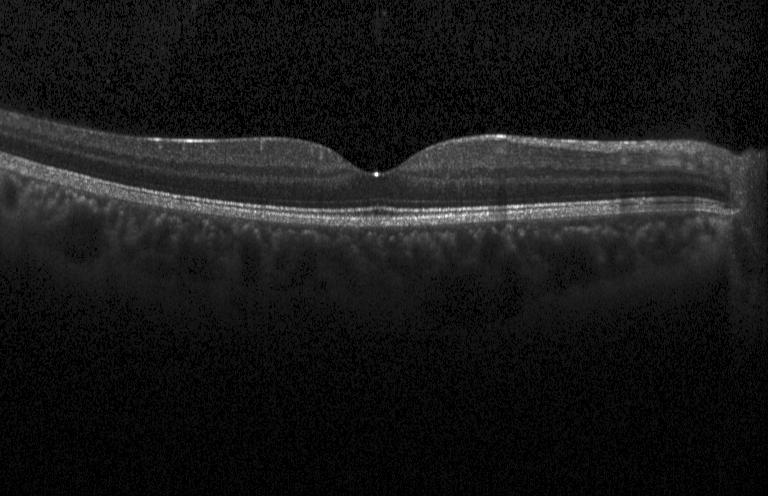 Fovea-centered. Optical coherence tomography B-scan. Spectral-domain OCT.
Finding: neither CNV, DME, nor drusen.